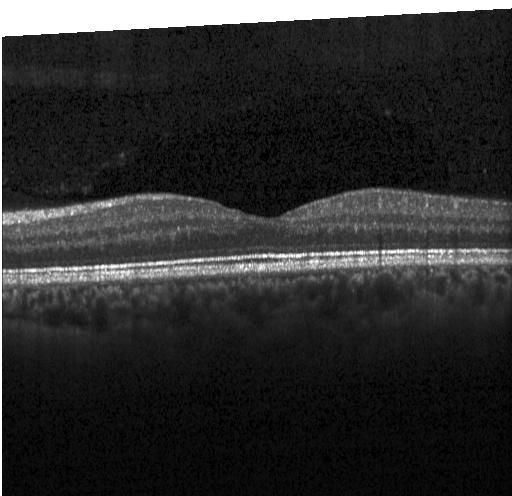
Impression: no CNV, DME, or drusen.